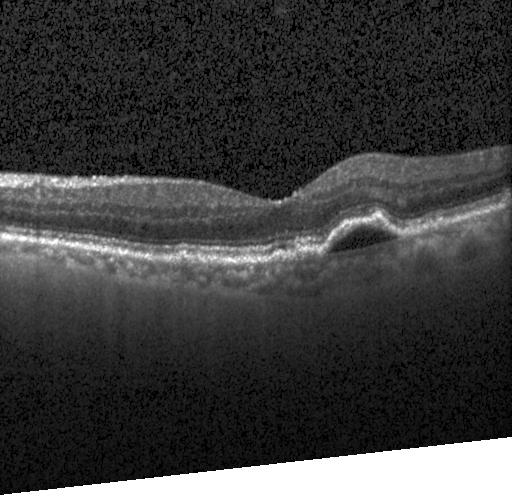

Retinal OCT cross-section; fovea-centered; SD-OCT
Macular OCT: a choroidal neovascular membrane.